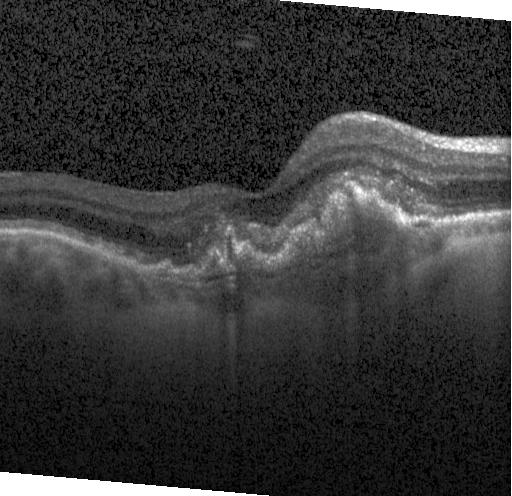

Optical coherence tomography scan. A choroidal neovascular membrane.